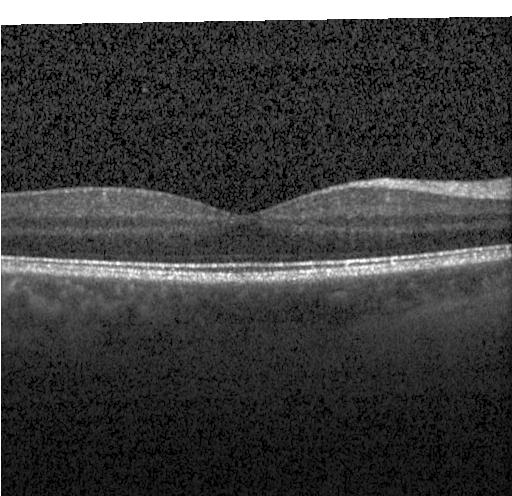

Diagnosis: no choroidal neovascularization, no diabetic macular edema, and no drusen.